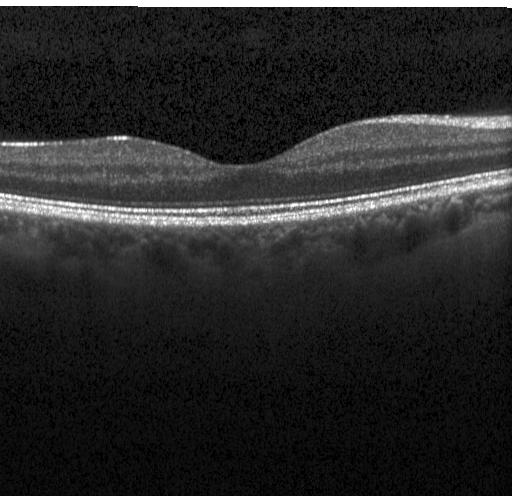 SD-OCT; acquired on a Heidelberg Spectralis; OCT line scan. Neither choroidal neovascularization, diabetic macular edema, nor drusen.